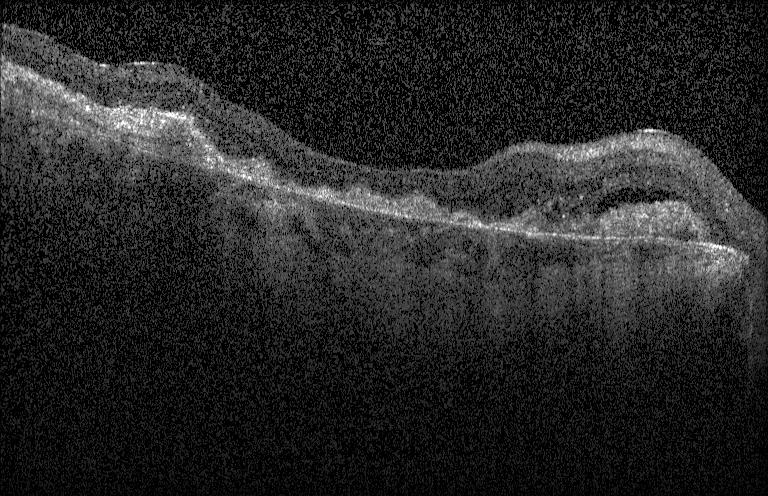 Heidelberg Spectralis. Retinal OCT cross-section. SD-OCT
The scan shows choroidal neovascularization (CNV).